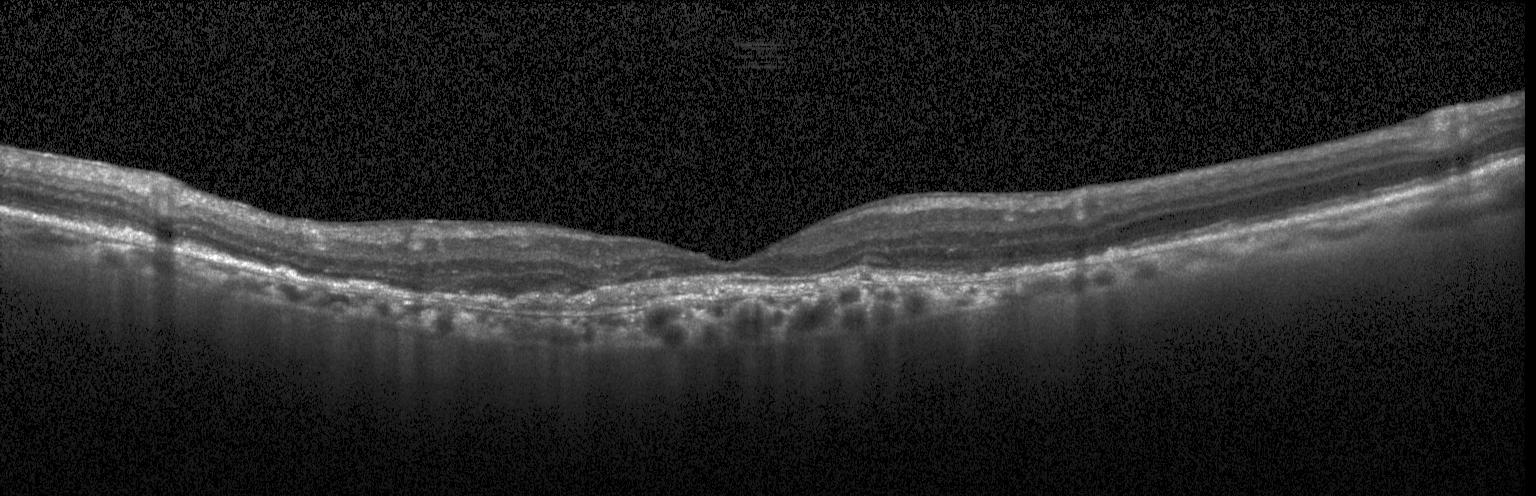

The scan shows choroidal neovascularization.